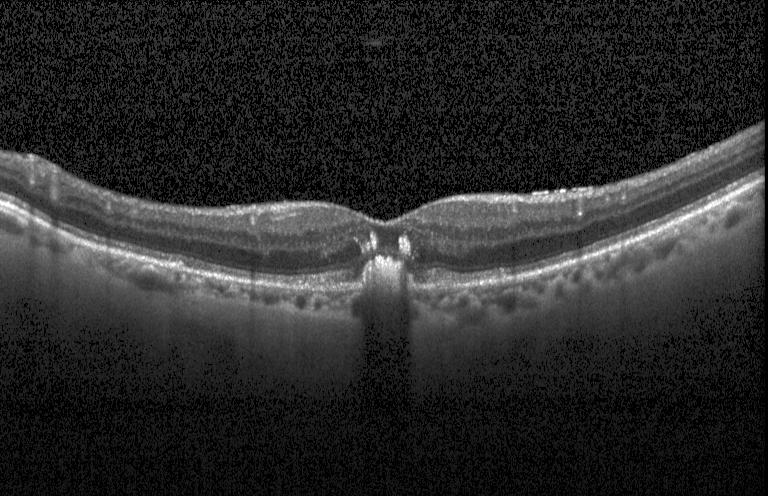 This B-scan demonstrates a choroidal neovascular membrane.